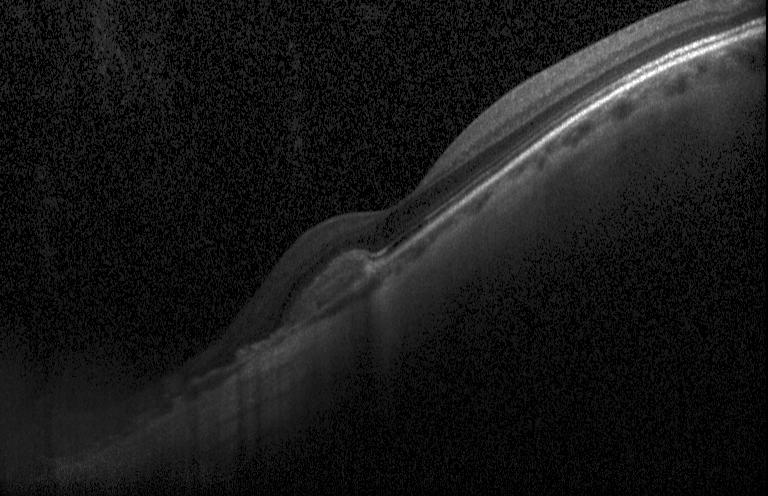 Retinal OCT cross-section showing a choroidal neovascular membrane.